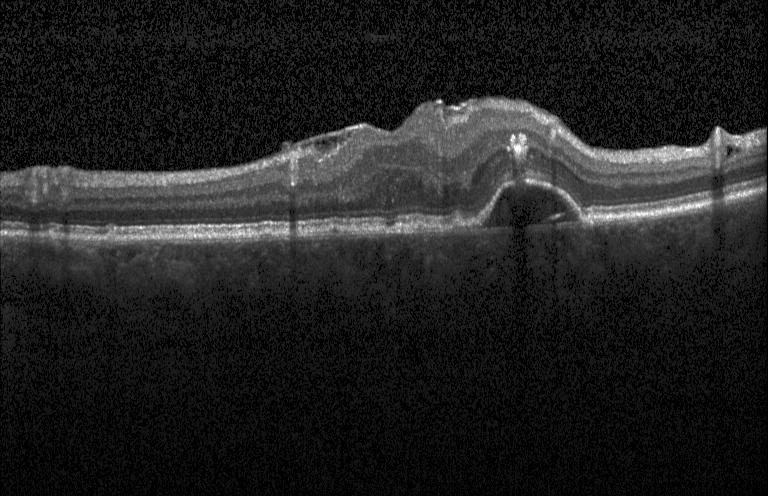 Finding: a choroidal neovascular membrane.